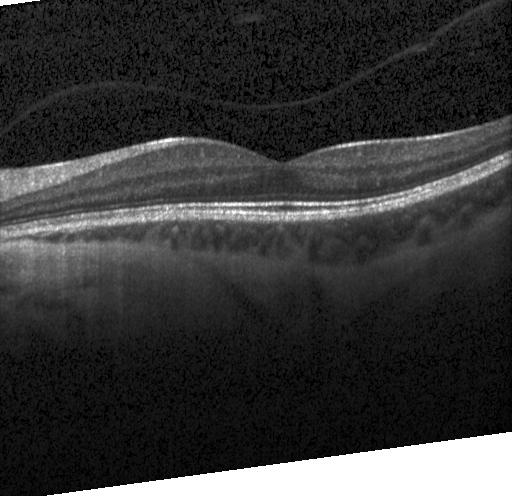

Optical coherence tomography B-scan — Diagnosis: no choroidal neovascularization, no diabetic macular edema, and no drusen.